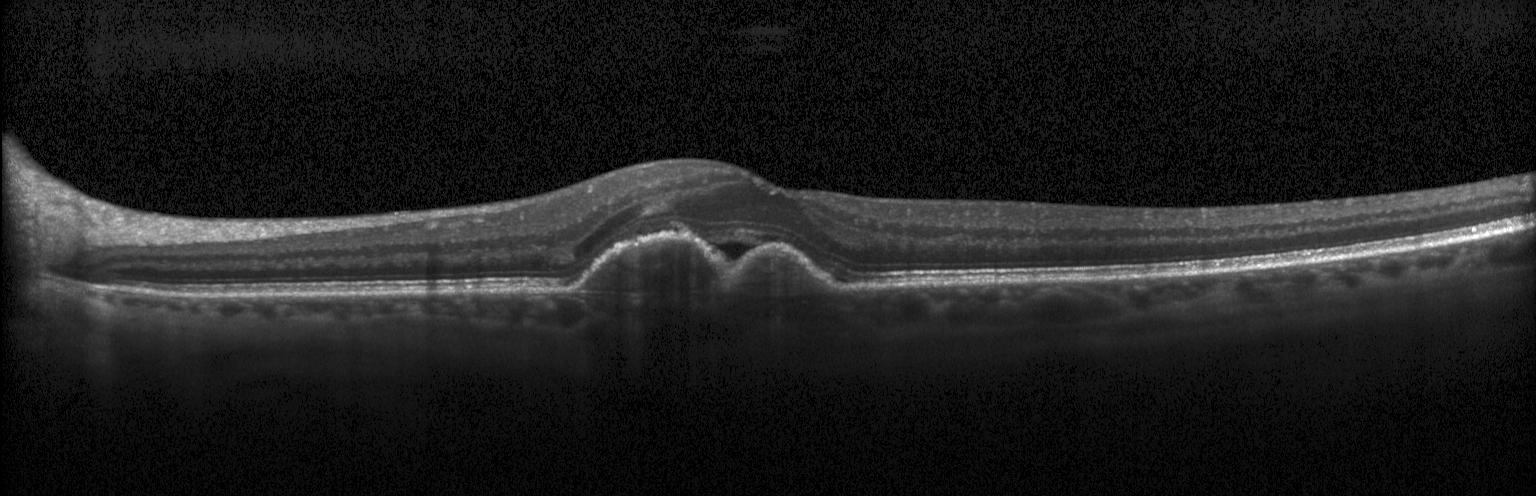 Heidelberg Spectralis OCT system · SD-OCT · retinal OCT B-scan. Diagnosis: a choroidal neovascular membrane.